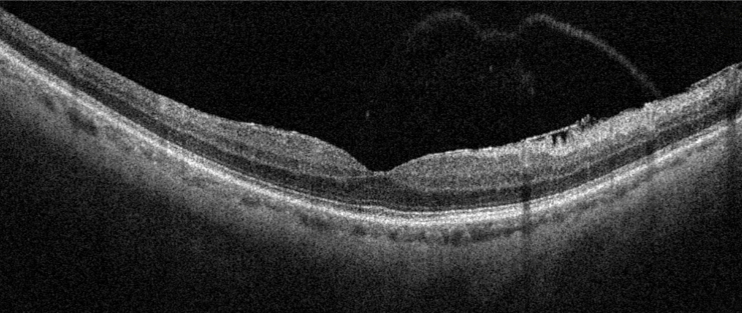
The scan shows epiretinal membrane (ERM).